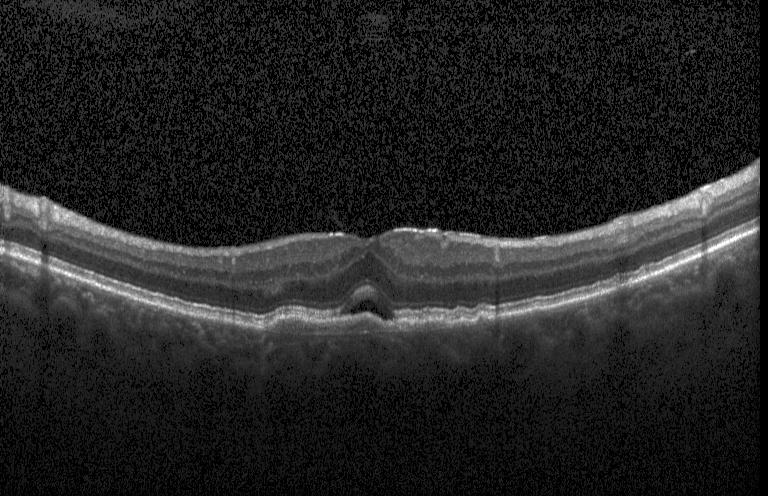

Macular scan; OCT B-scan; spectral-domain OCT; instrument: Heidelberg Spectralis — Diagnosis: a choroidal neovascular membrane.